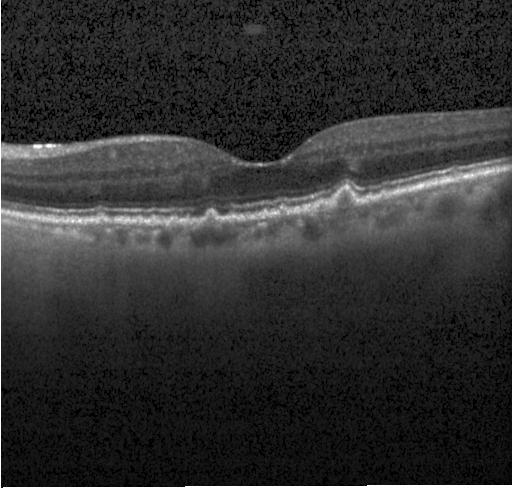
OCT line scan — Finding: multiple drusen.